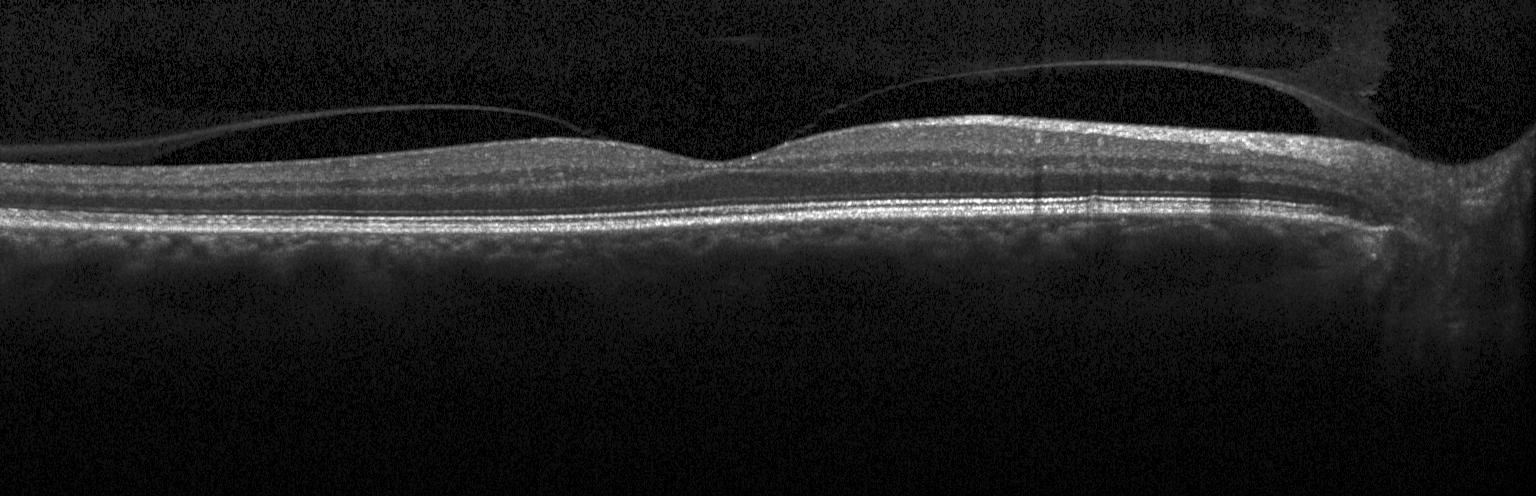
The scan shows no choroidal neovascularization, no diabetic macular edema, and no drusen.